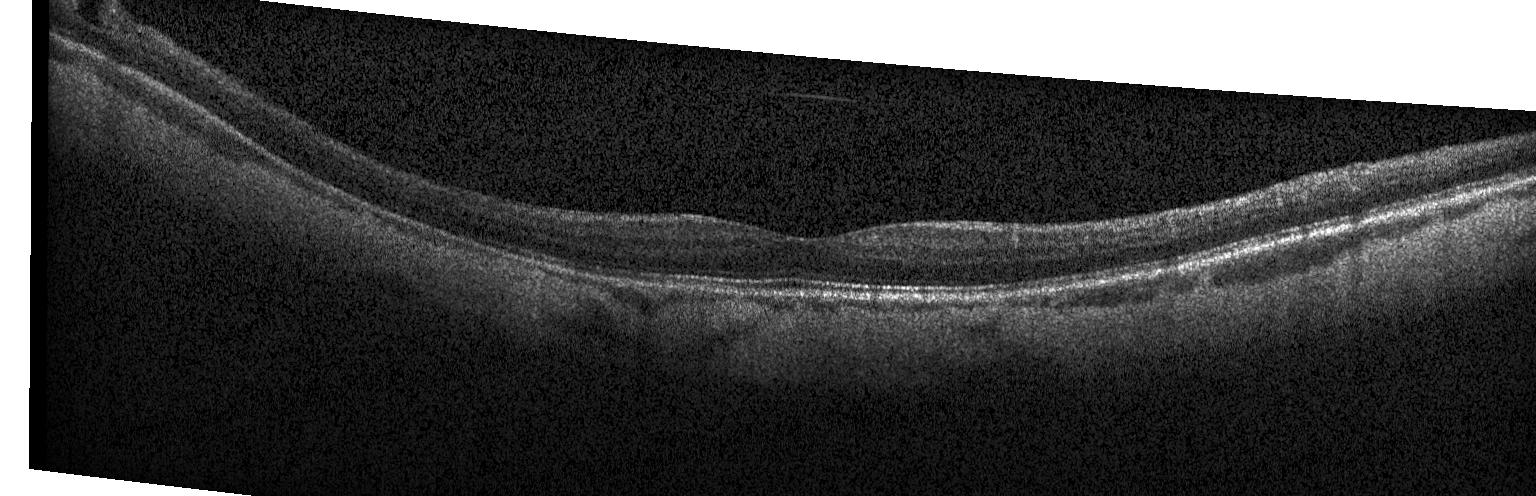 OCT line scan
This B-scan demonstrates no CNV, DME, or drusen.